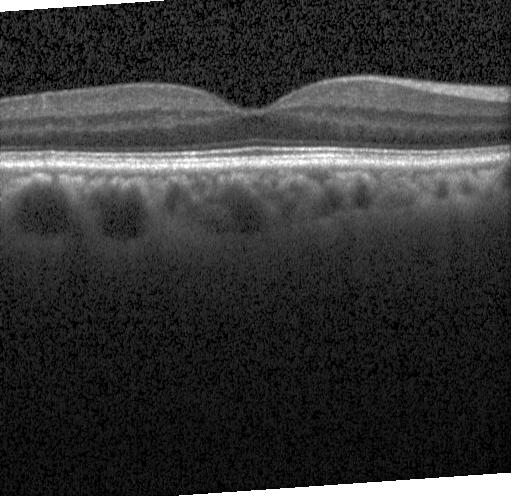
Optical coherence tomography B-scan. Instrument: Heidelberg Spectralis. Centered on the fovea. SD-OCT
No choroidal neovascularization, diabetic macular edema, or drusen.